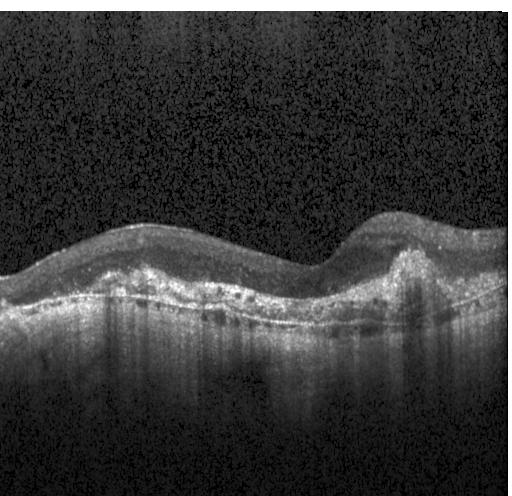 Optical coherence tomography scan.
Assessment: choroidal neovascularization (CNV).